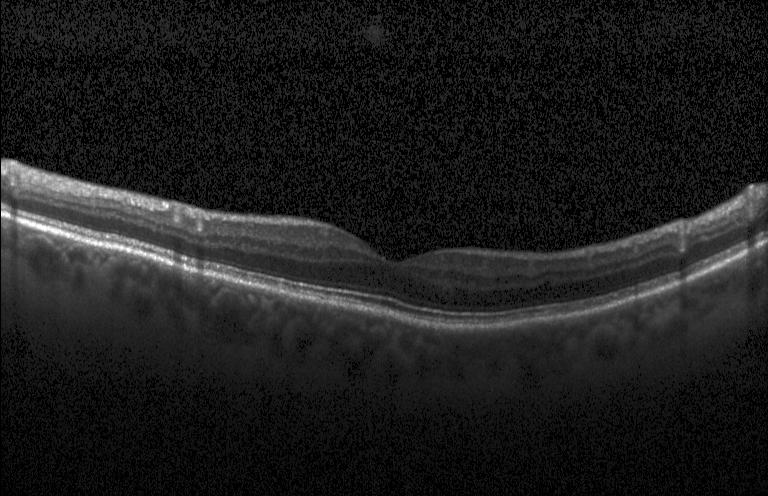 Optical coherence tomography B-scan — No choroidal neovascularization, no diabetic macular edema, and no drusen.